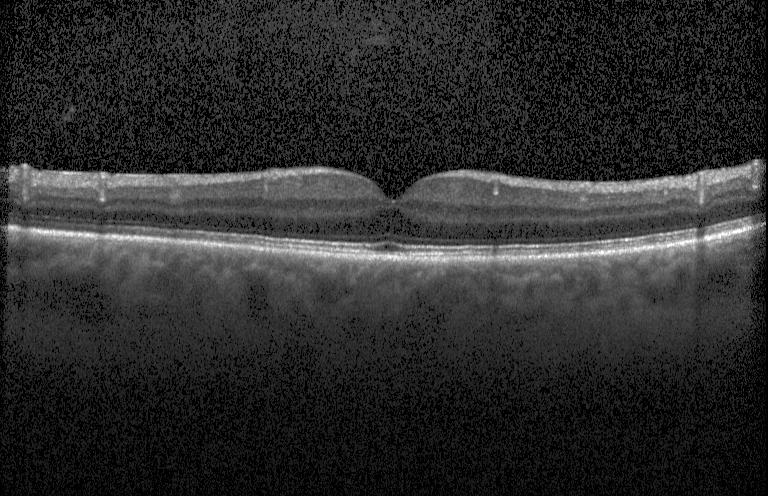 Retinal OCT cross-section showing no choroidal neovascularization, no diabetic macular edema, and no drusen.